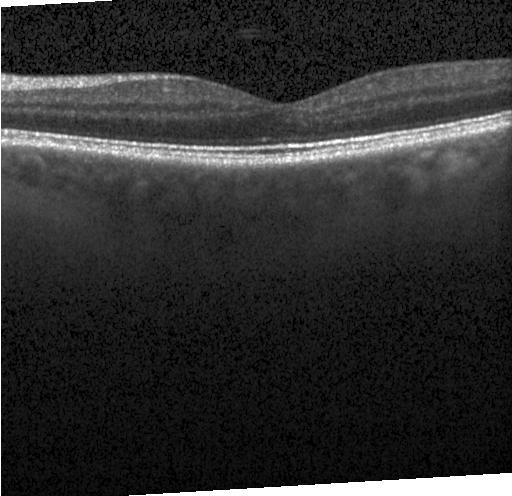 OCT finding: neither choroidal neovascularization, diabetic macular edema, nor drusen.